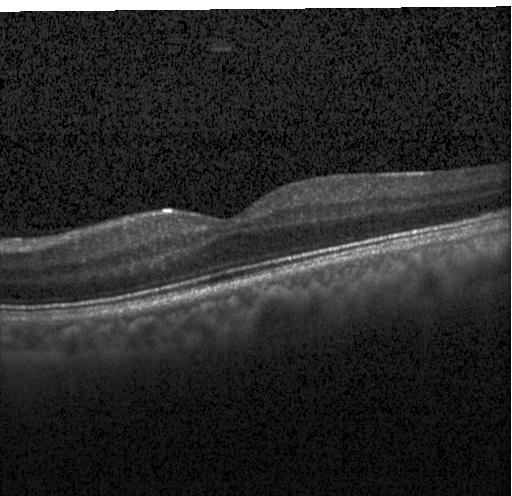
Optical coherence tomography B-scan, Heidelberg Spectralis OCT system, macular scan, spectral-domain optical coherence tomography.
OCT finding: no CNV, DME, or drusen.